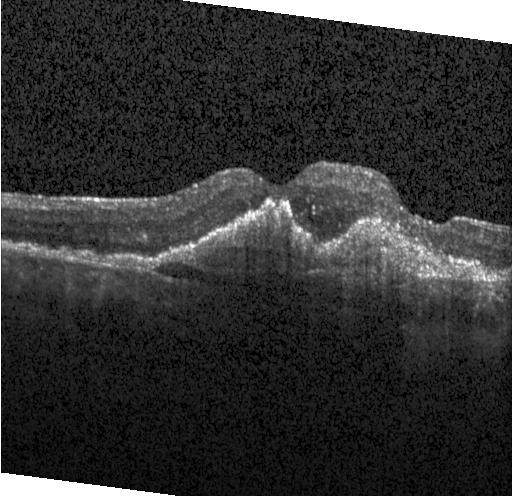 OCT line scan · SD-OCT
The scan shows choroidal neovascularization.